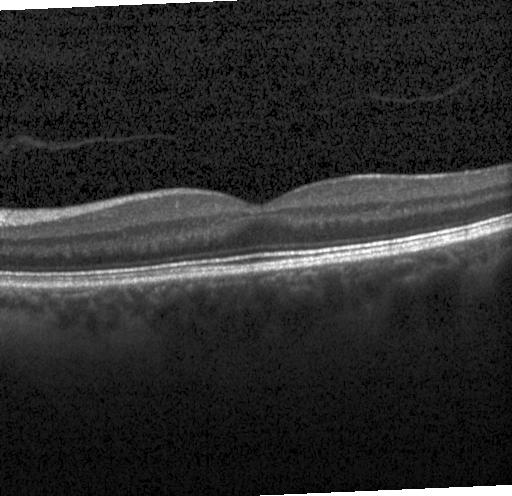

OCT line scan · Heidelberg Spectralis OCT system · SD-OCT · fovea-centered.
Assessment: no choroidal neovascularization, no diabetic macular edema, and no drusen.